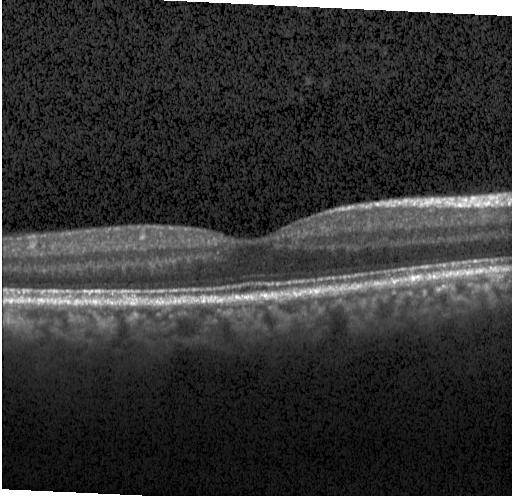
Optical coherence tomography scan
Assessment: neither CNV, DME, nor drusen.